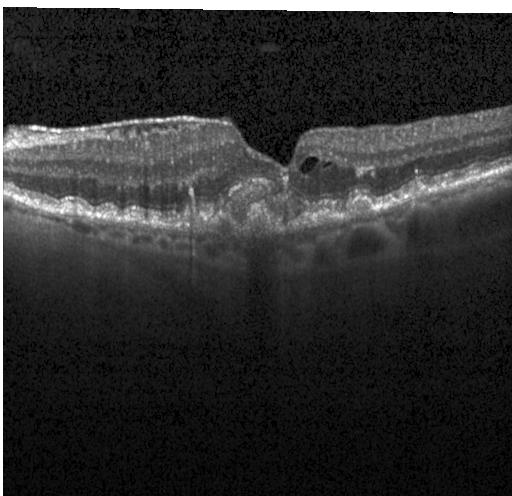

OCT line scan · spectral-domain OCT · Heidelberg Spectralis OCT system
This B-scan demonstrates a choroidal neovascular membrane.